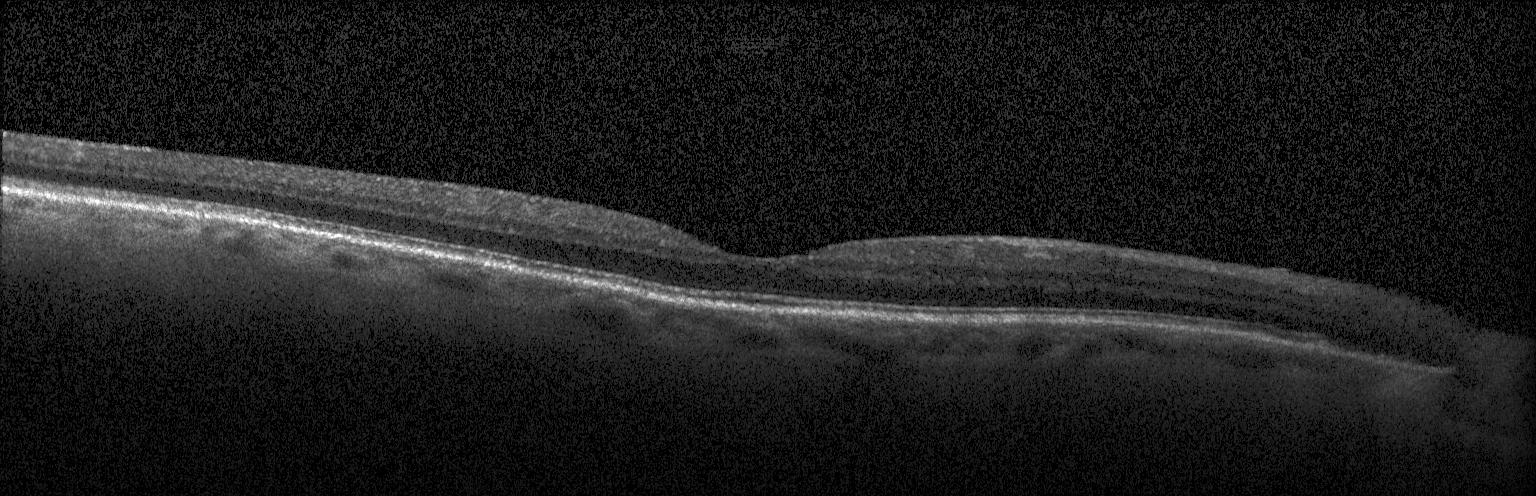 Optical coherence tomography scan — Diagnosis: no choroidal neovascularization, diabetic macular edema, or drusen.